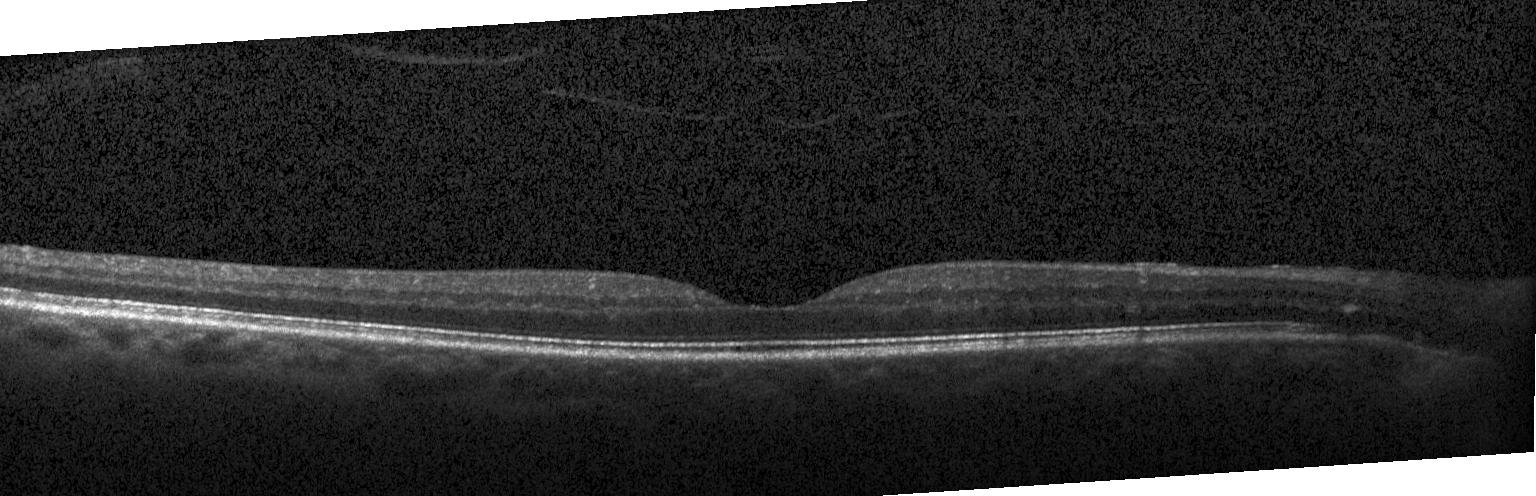 Acquired on a Heidelberg Spectralis · retinal OCT B-scan · spectral-domain optical coherence tomography · fovea-centered.
Impression: no choroidal neovascularization, no diabetic macular edema, and no drusen.